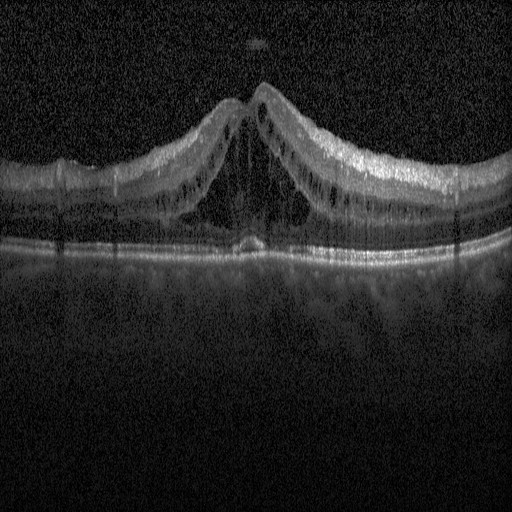 Retinal OCT cross-section
Diabetic macular edema.